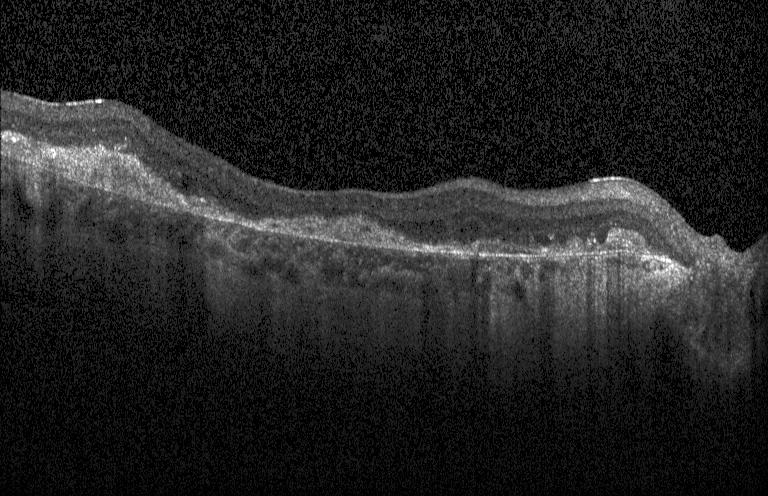 Centered on the fovea. Spectral-domain optical coherence tomography. Retinal OCT B-scan.
Diagnosis: CNV.